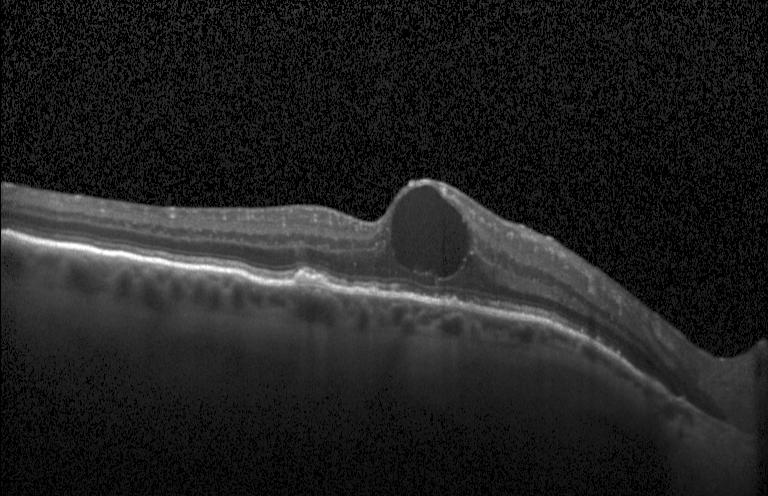
Retinal OCT B-scan — The scan shows choroidal neovascularization (CNV).